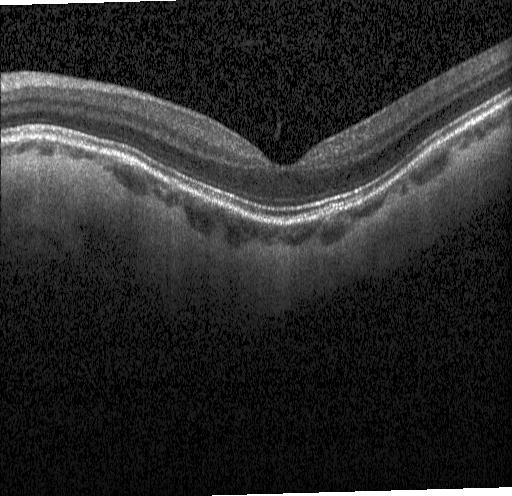

Dx: no evidence of CNV, DME, or drusen.